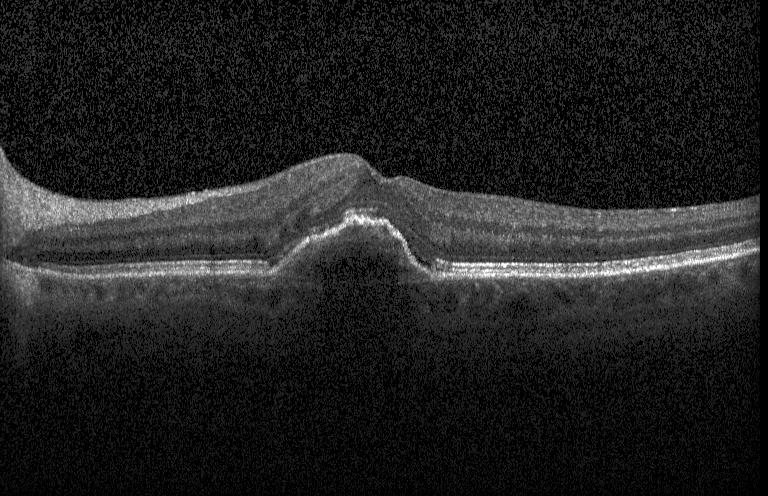 Retinal OCT cross-section — Impression: choroidal neovascularization.